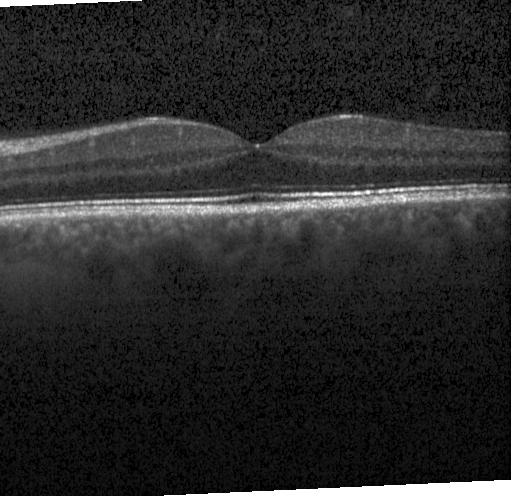
Horizontal scan through the fovea · spectral-domain OCT · acquired on a Heidelberg Spectralis · retinal OCT B-scan.
Assessment: no choroidal neovascularization, diabetic macular edema, or drusen.